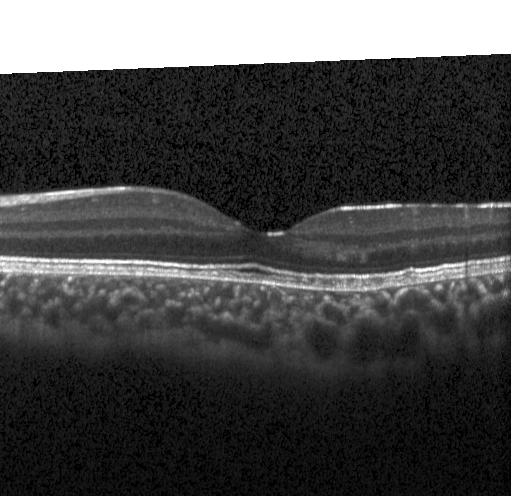 Horizontal scan through the fovea; Heidelberg Spectralis OCT system; OCT B-scan
Impression: no CNV, DME, or drusen.